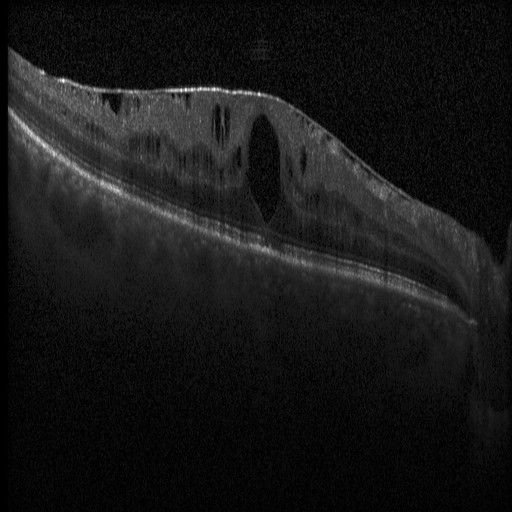
Impression: diabetic macular edema (DME).